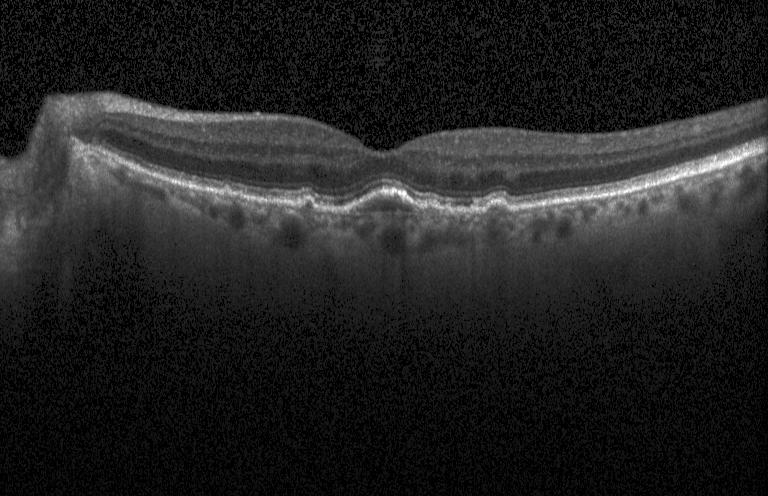

Acquired on a Heidelberg Spectralis, OCT line scan. Macular OCT: choroidal neovascularization.